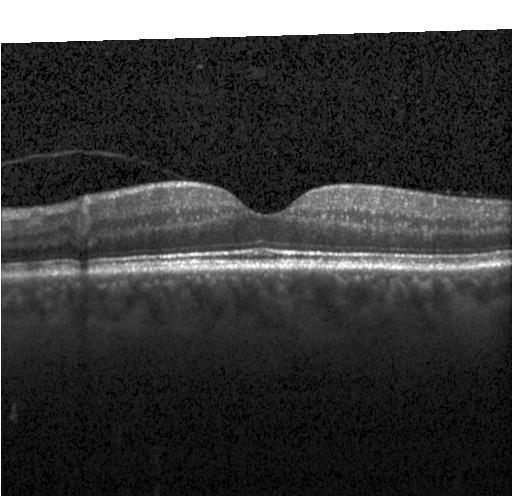 Macular OCT demonstrating no evidence of choroidal neovascularization, diabetic macular edema, or drusen.